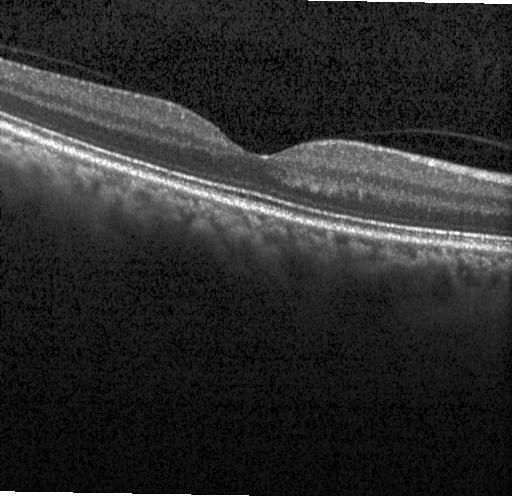
Macular scan, optical coherence tomography B-scan, Heidelberg Spectralis OCT system
No choroidal neovascularization, no diabetic macular edema, and no drusen.